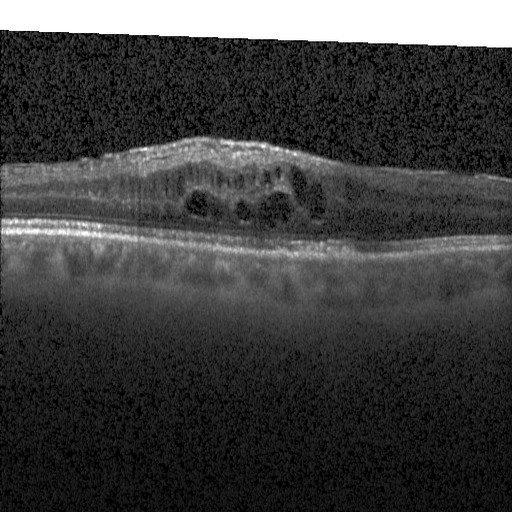 Spectral-domain OCT B-scan: diabetic macular edema.